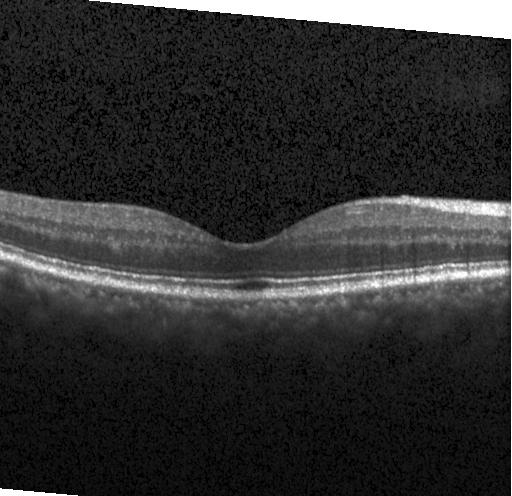 Retinal OCT B-scan, acquired on a Heidelberg Spectralis, through the macula
This B-scan demonstrates no evidence of CNV, DME, or drusen.